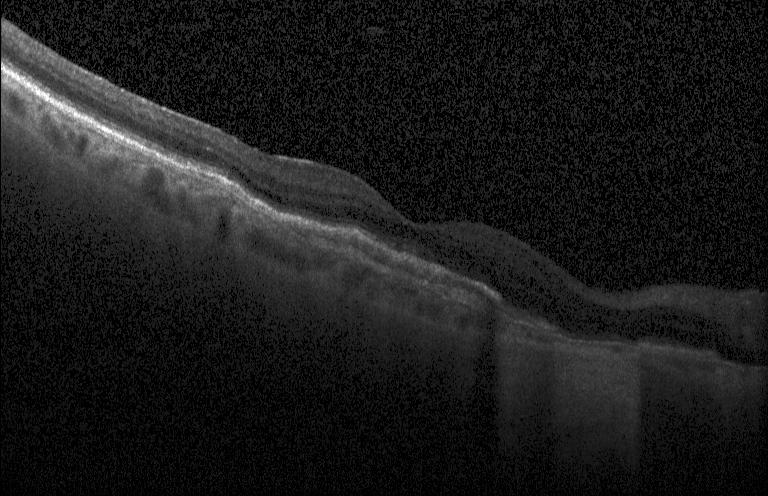 Acquired on a Heidelberg Spectralis · optical coherence tomography B-scan · through the macula · spectral-domain OCT. Impression: choroidal neovascularization.